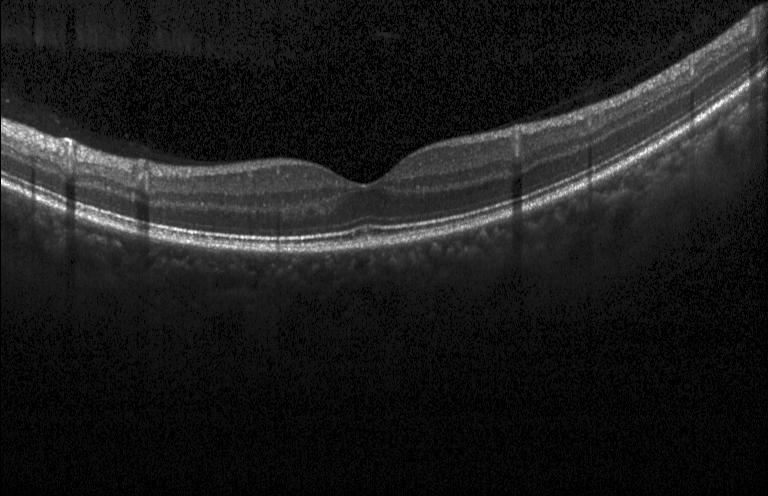 Instrument: Heidelberg Spectralis. OCT line scan. Spectral-domain OCT. Horizontal scan through the fovea
Finding: no evidence of choroidal neovascularization, diabetic macular edema, or drusen.